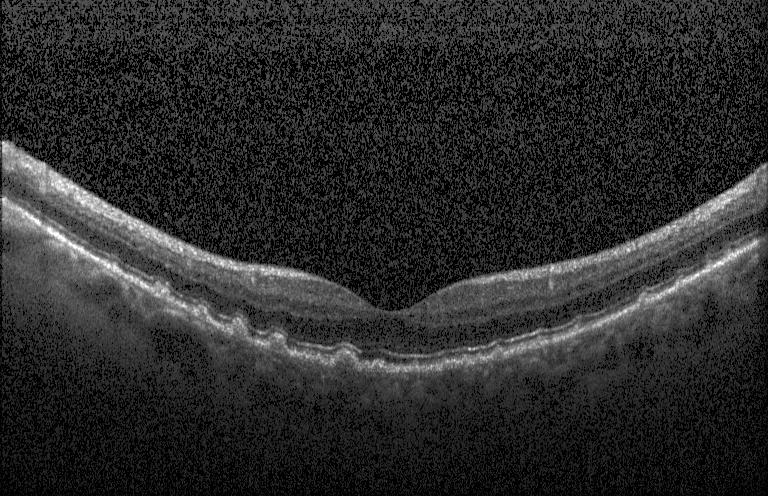 OCT finding: sub-RPE drusenoid deposits.